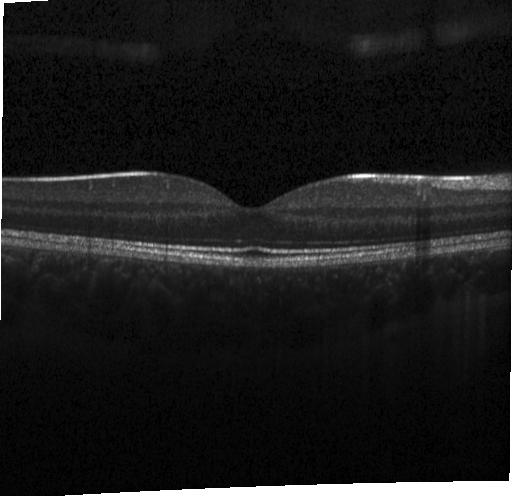

Spectral-domain OCT B-scan: no evidence of choroidal neovascularization, diabetic macular edema, or drusen.